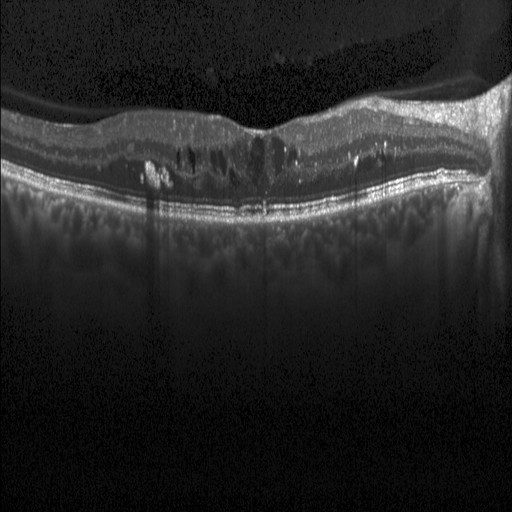

Retinal OCT B-scan — This B-scan demonstrates diabetic macular edema (DME).